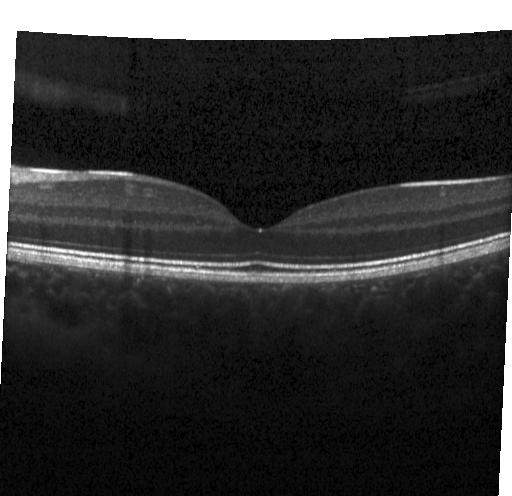 OCT scan showing no CNV, no DME, and no drusen.